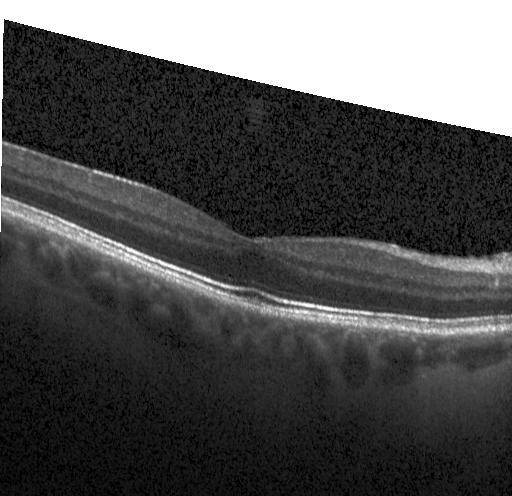
Dx: no choroidal neovascularization, no diabetic macular edema, and no drusen.